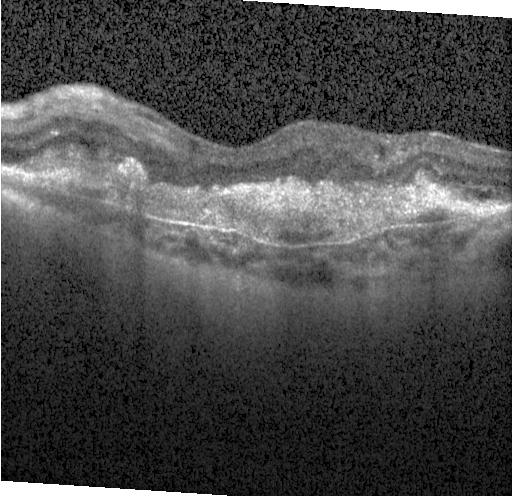
Heidelberg Spectralis; macular scan; spectral-domain optical coherence tomography; retinal OCT cross-section
Finding: a choroidal neovascular membrane.